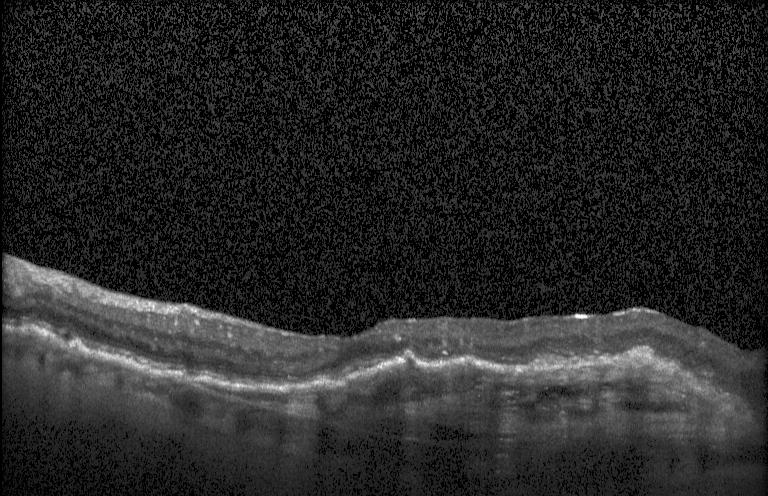

Instrument: Heidelberg Spectralis · OCT B-scan · through the macula. Impression: choroidal neovascularization (CNV).